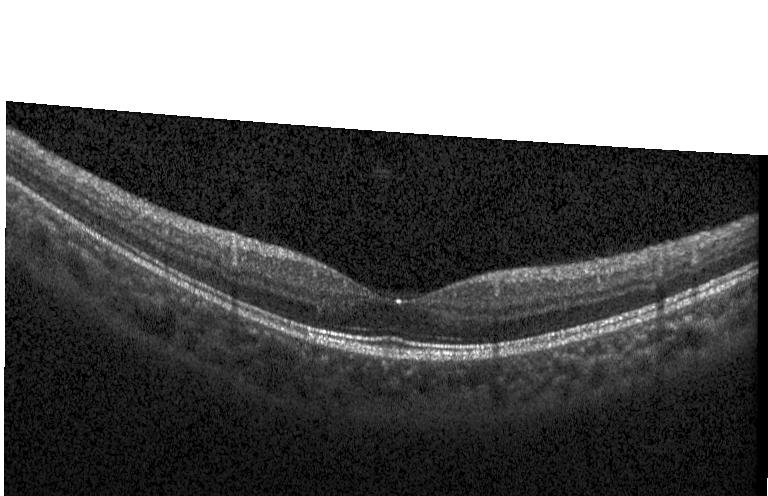

Centered on the fovea, spectral-domain optical coherence tomography, optical coherence tomography scan
Macular OCT: no CNV, no DME, and no drusen.